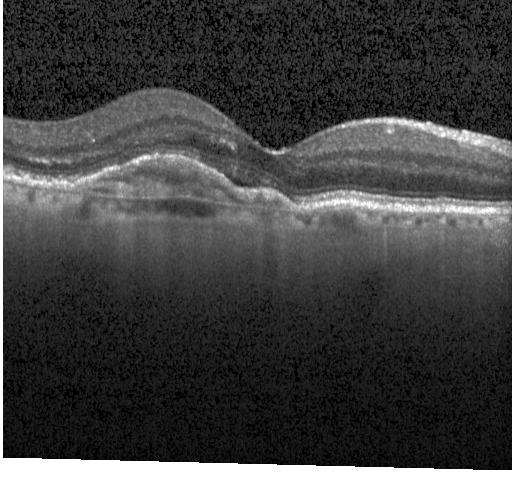 Centered on the fovea · optical coherence tomography scan · SD-OCT · Heidelberg Spectralis
The scan shows CNV.